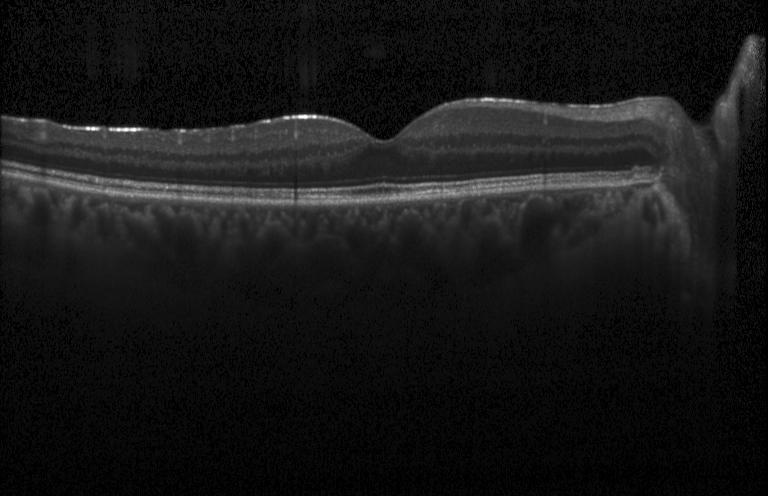 Centered on the fovea; optical coherence tomography scan.
Impression: neither choroidal neovascularization, diabetic macular edema, nor drusen.